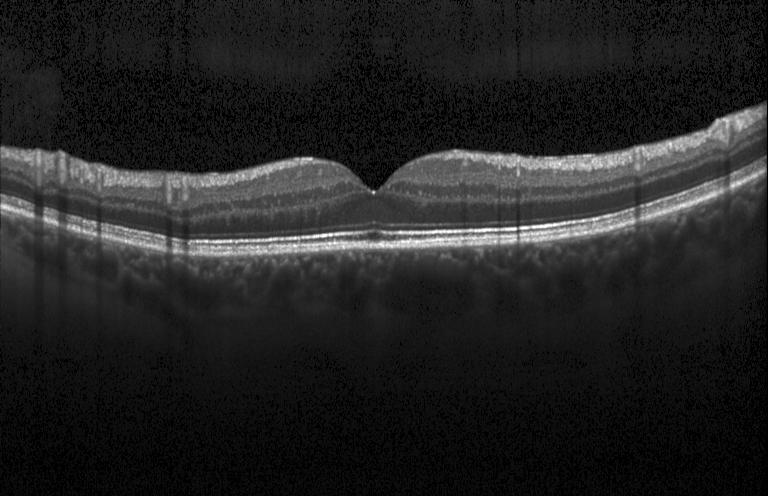

Finding: no CNV, DME, or drusen.